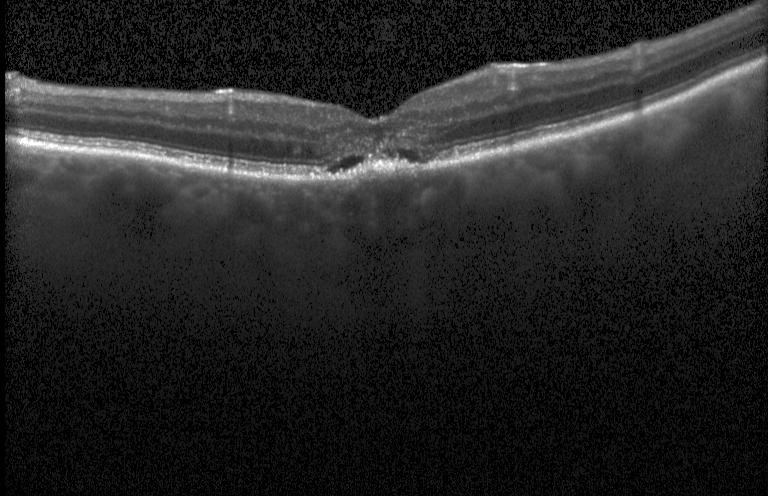
Fovea-centered · optical coherence tomography B-scan.
Finding: a choroidal neovascular membrane.